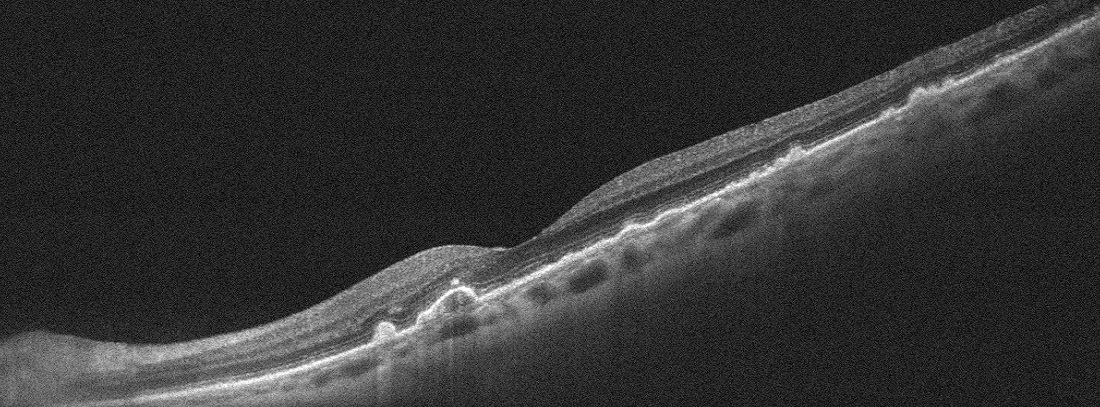

OCT finding: AMD.